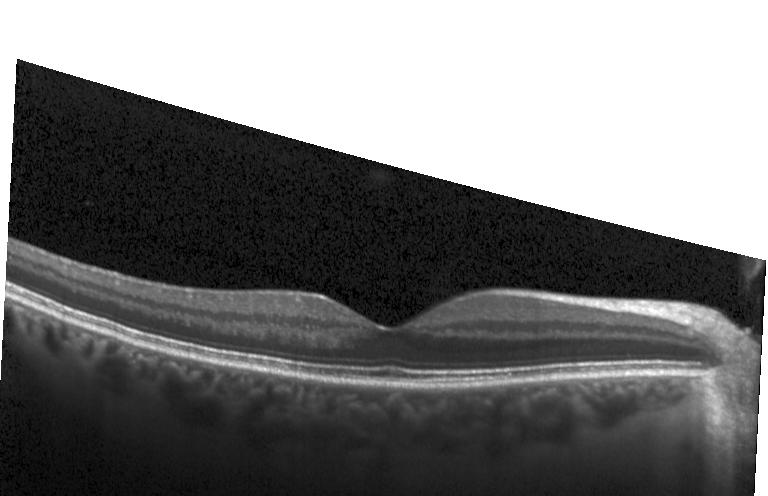
Diagnosis: no choroidal neovascularization, no diabetic macular edema, and no drusen.